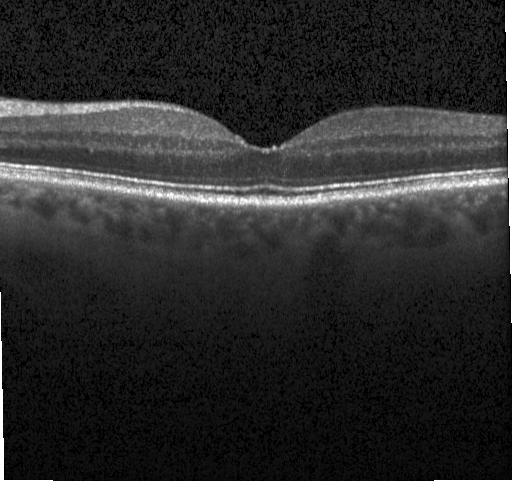 Macular scan, OCT line scan, spectral-domain optical coherence tomography.
Impression: no evidence of choroidal neovascularization, diabetic macular edema, or drusen.